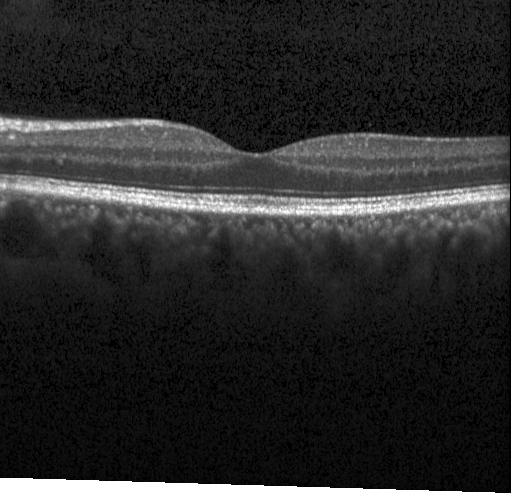

Instrument: Heidelberg Spectralis · optical coherence tomography B-scan · centered on the fovea · spectral-domain OCT. Assessment: no evidence of choroidal neovascularization, diabetic macular edema, or drusen.